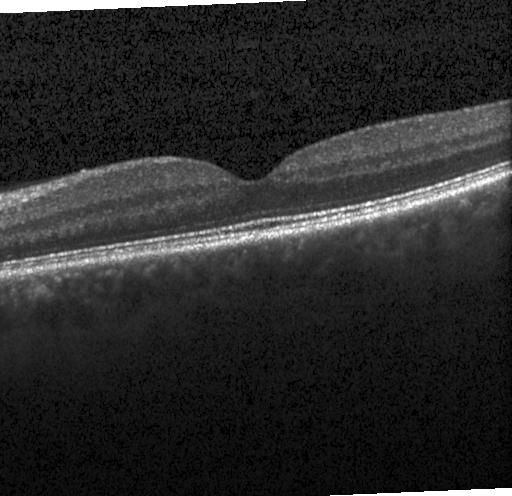 OCT line scan. Acquired on a Heidelberg Spectralis. SD-OCT. Macular scan — Assessment: neither choroidal neovascularization, diabetic macular edema, nor drusen.